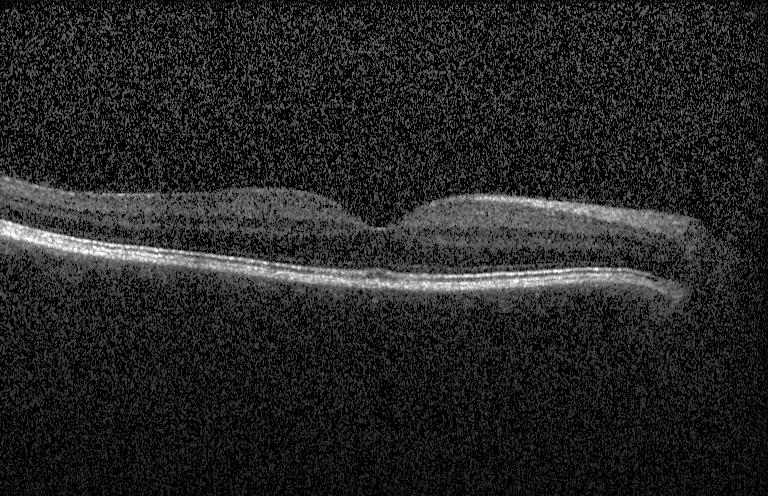 OCT B-scan; spectral-domain OCT; instrument: Heidelberg Spectralis; through the macula — The scan shows no evidence of choroidal neovascularization, diabetic macular edema, or drusen.